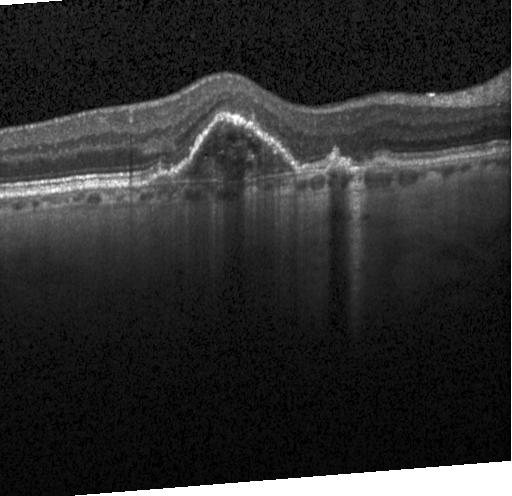
Macular OCT: choroidal neovascularization (CNV).